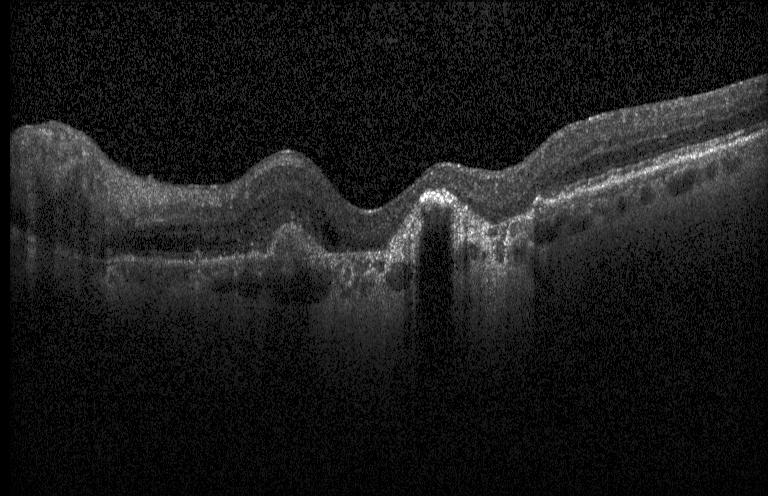
Impression: choroidal neovascularization (CNV).